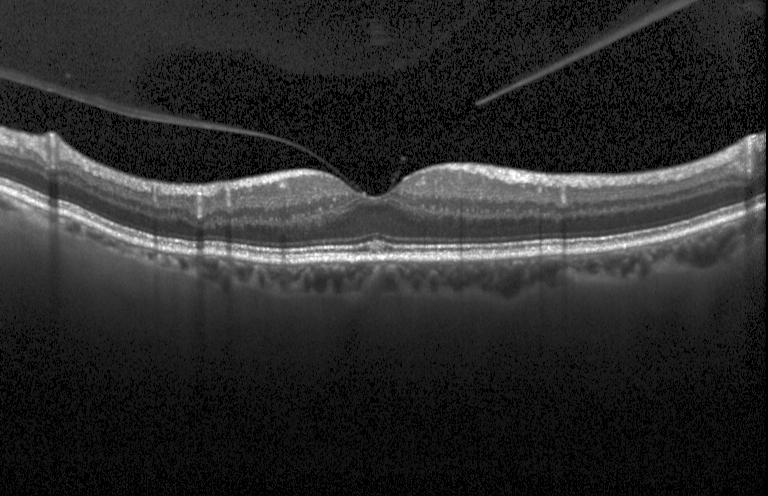
OCT B-scan · SD-OCT · fovea-centered. The scan shows neither choroidal neovascularization, diabetic macular edema, nor drusen.